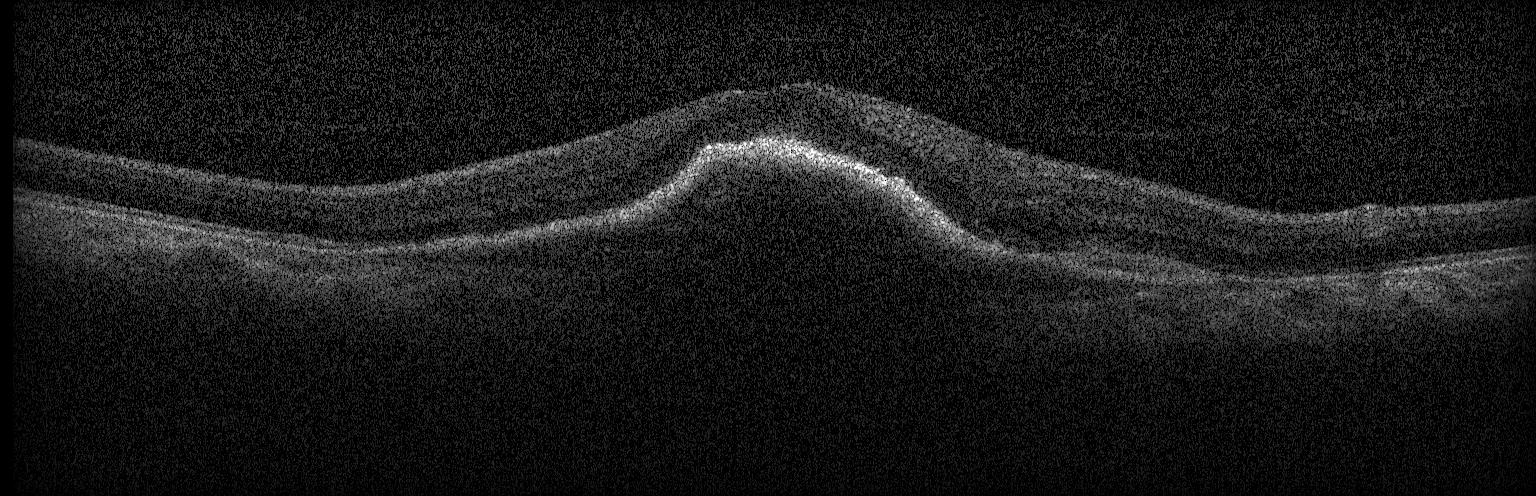 Assessment: CNV.